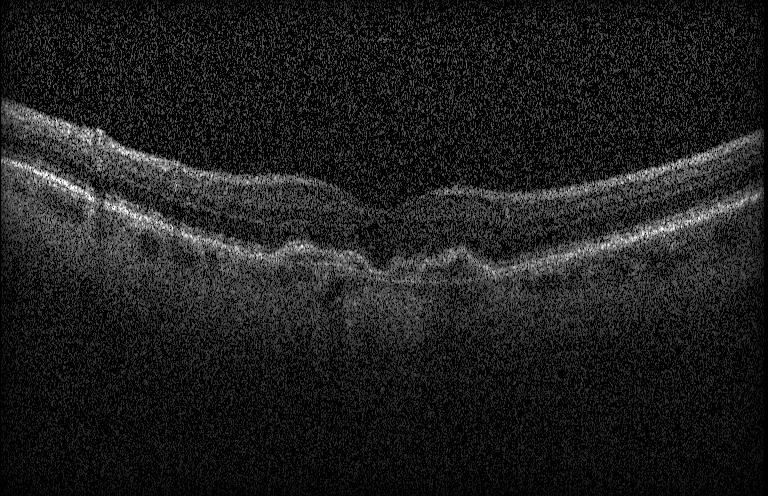 Optical coherence tomography scan. OCT finding: a choroidal neovascular membrane.